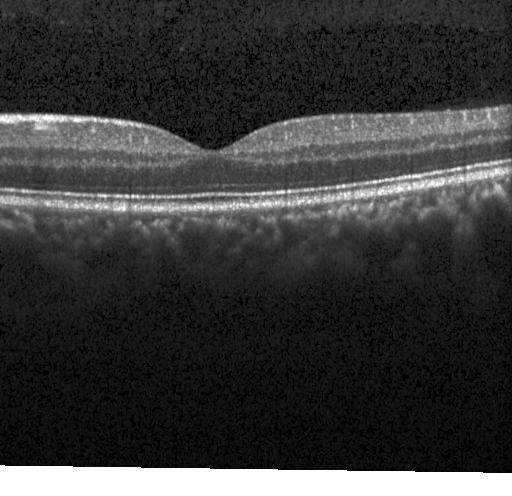

Optical coherence tomography scan. Through the macula. Heidelberg Spectralis OCT system. SD-OCT — Macular OCT: neither CNV, DME, nor drusen.